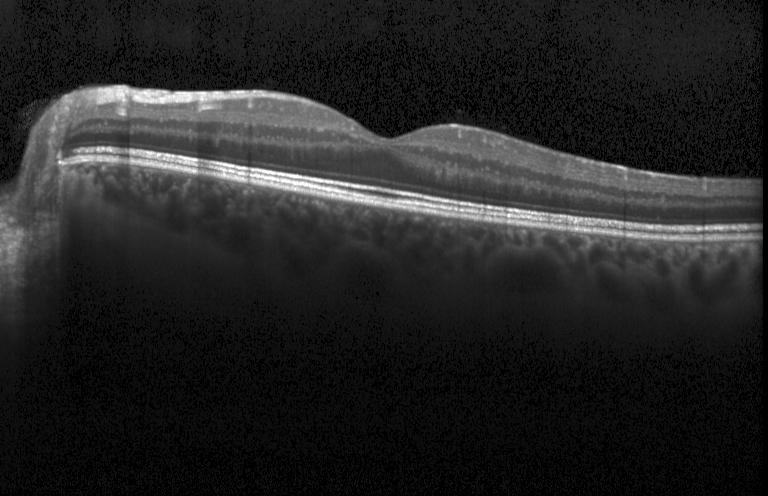

OCT finding: no choroidal neovascularization, diabetic macular edema, or drusen.